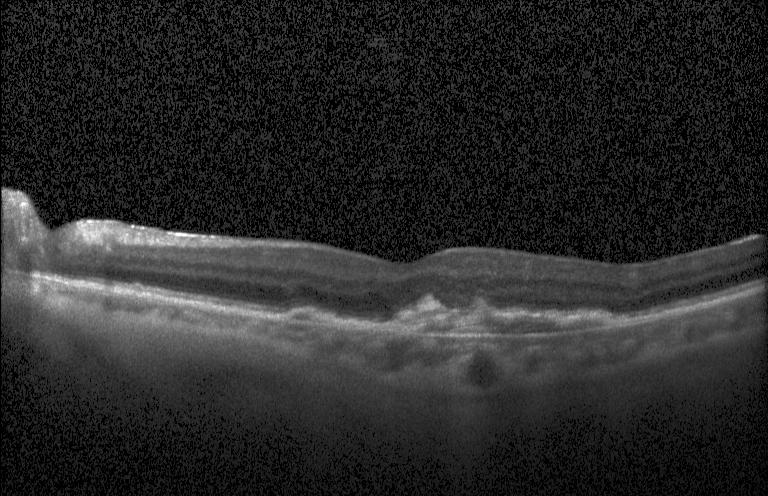 Spectral-domain OCT; macular scan; optical coherence tomography scan; Heidelberg Spectralis
The scan shows CNV.